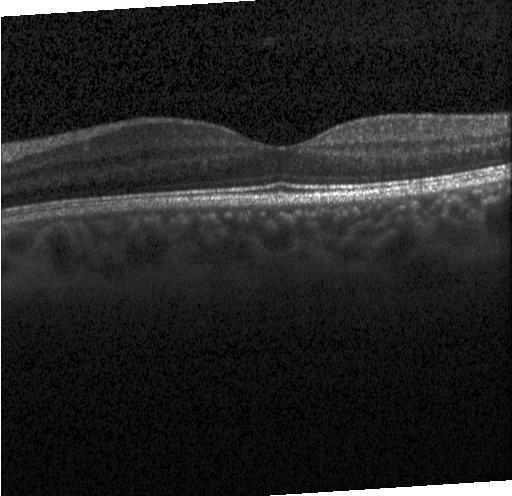

Finding: no choroidal neovascularization, diabetic macular edema, or drusen.